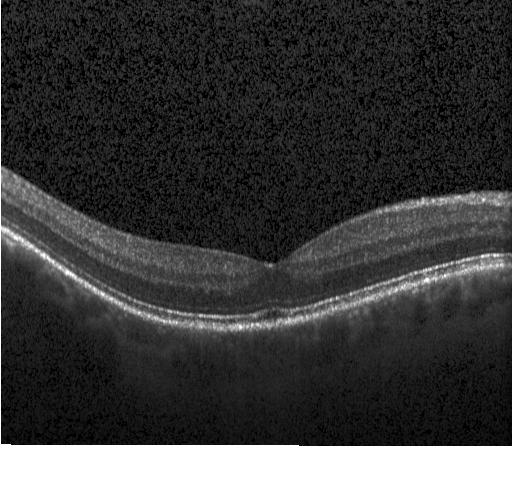

Optical coherence tomography scan. Diagnosis: neither CNV, DME, nor drusen.